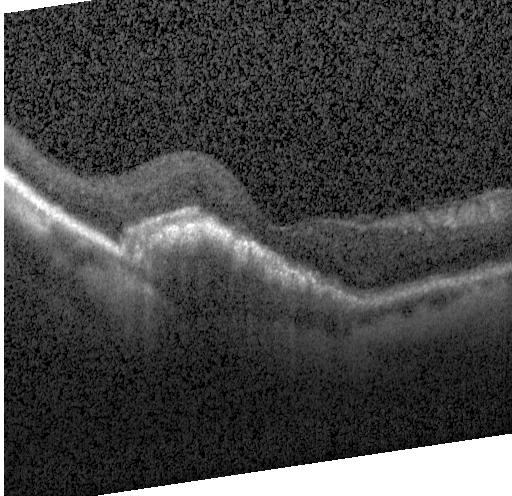

Finding: CNV.